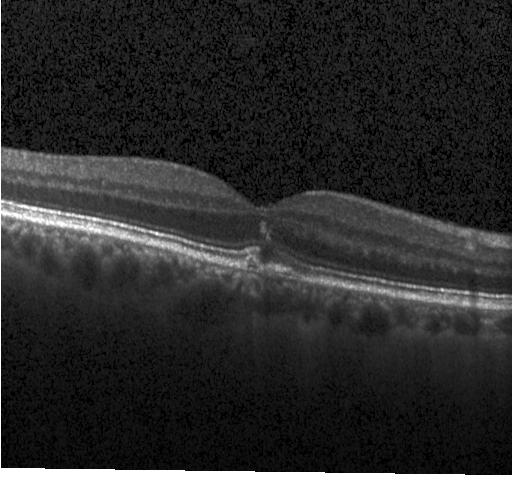 Retinal OCT cross-section. Assessment: a choroidal neovascular membrane.